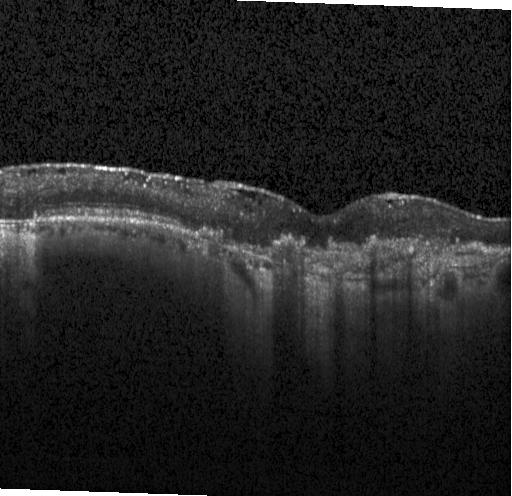
Finding: choroidal neovascularization (CNV).